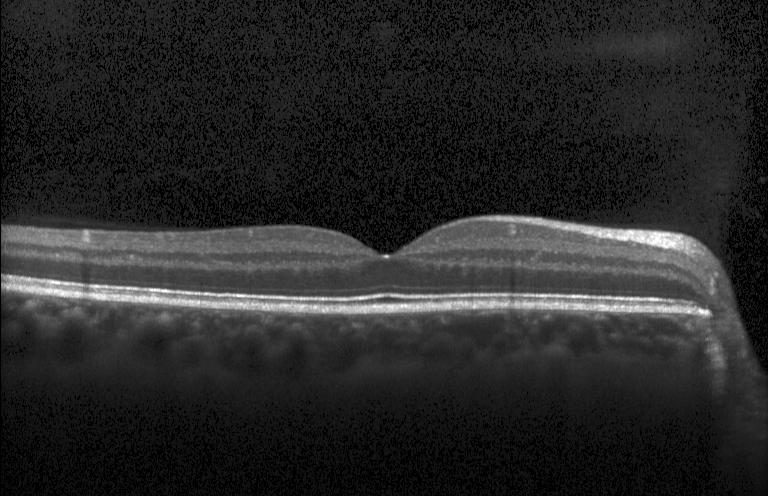

Optical coherence tomography B-scan. Horizontal scan through the fovea. SD-OCT
Dx: no choroidal neovascularization, no diabetic macular edema, and no drusen.